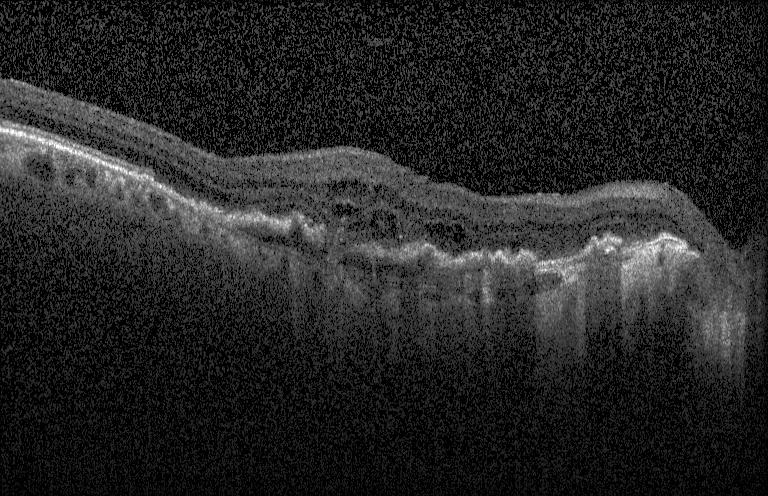

Retinal OCT B-scan. Centered on the fovea. Spectral-domain optical coherence tomography. Finding: a choroidal neovascular membrane.